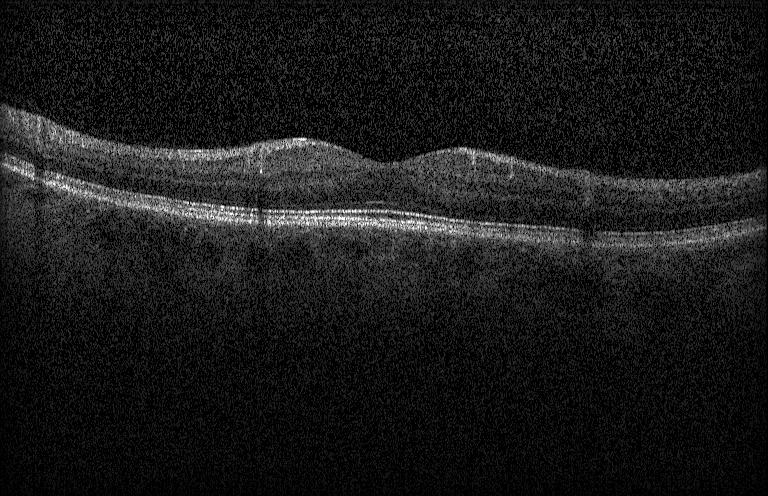
SD-OCT. Heidelberg Spectralis OCT system. Macular scan. Retinal OCT cross-section — Diagnosis: neither choroidal neovascularization, diabetic macular edema, nor drusen.